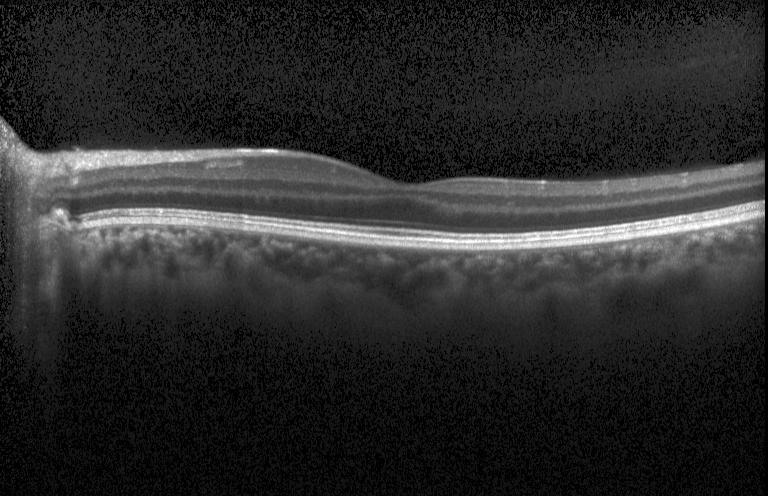

Optical coherence tomography scan.
Finding: no evidence of choroidal neovascularization, diabetic macular edema, or drusen.